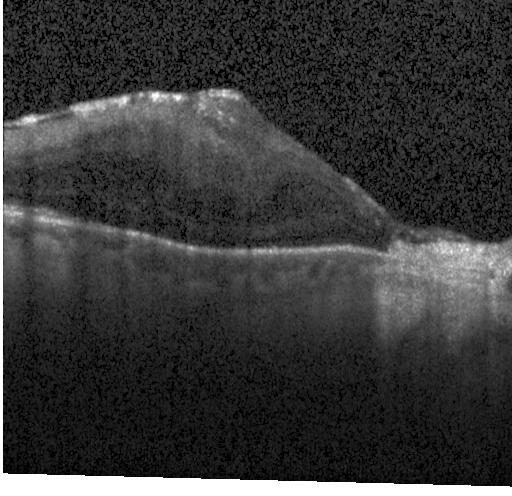
Assessment: diabetic macular edema (DME).